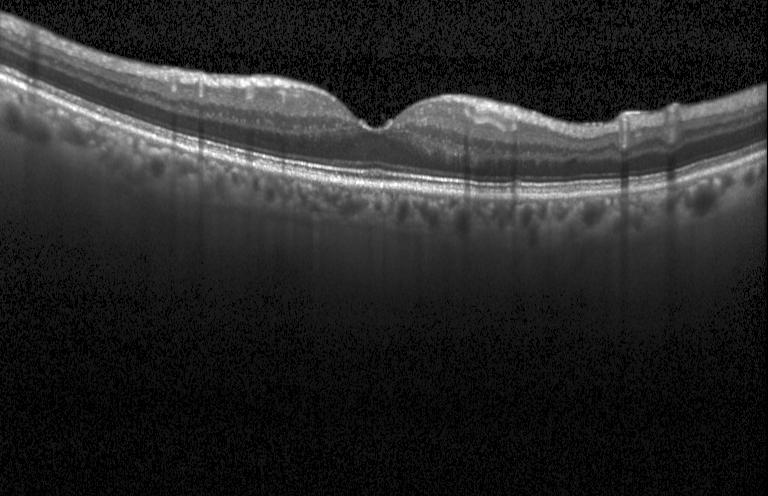

Through the macula · OCT line scan · spectral-domain optical coherence tomography
The scan shows no evidence of choroidal neovascularization, diabetic macular edema, or drusen.